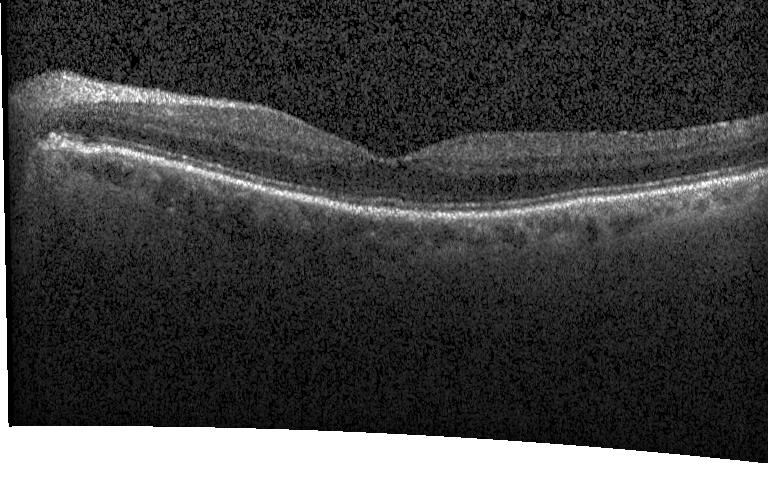

Heidelberg Spectralis OCT system. Retinal OCT cross-section. Spectral-domain optical coherence tomography.
Dx: no CNV, no DME, and no drusen.